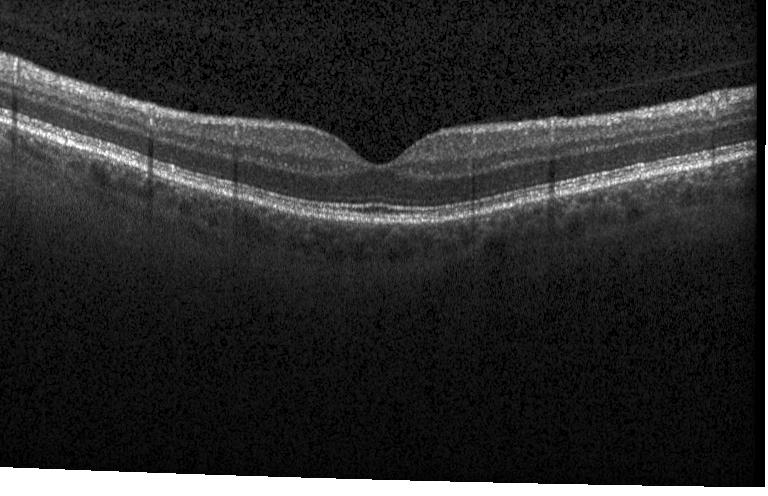 Centered on the fovea. Acquired on a Heidelberg Spectralis. Spectral-domain OCT. Retinal OCT cross-section — Assessment: no choroidal neovascularization, no diabetic macular edema, and no drusen.